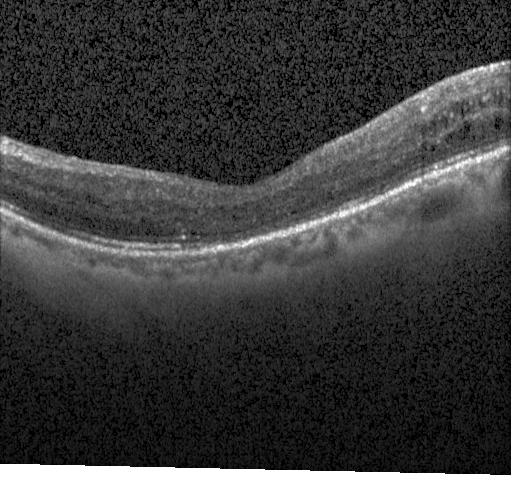
SD-OCT. Heidelberg Spectralis. Horizontal scan through the fovea. OCT B-scan.
The scan shows diabetic macular edema (DME).